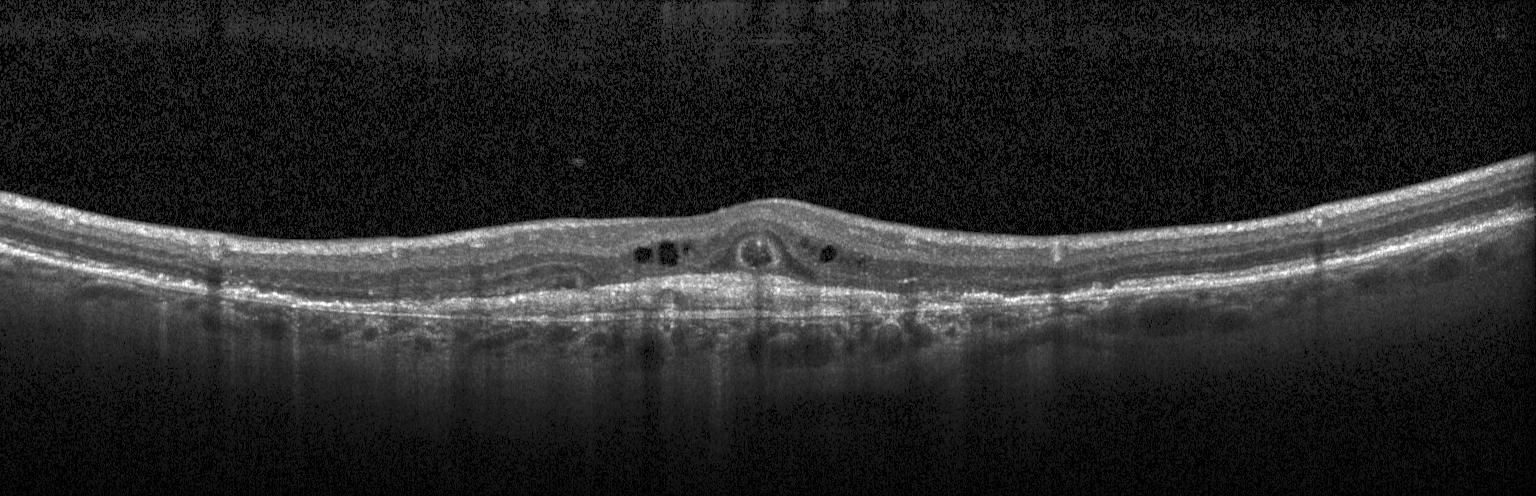
Diagnosis: a choroidal neovascular membrane.